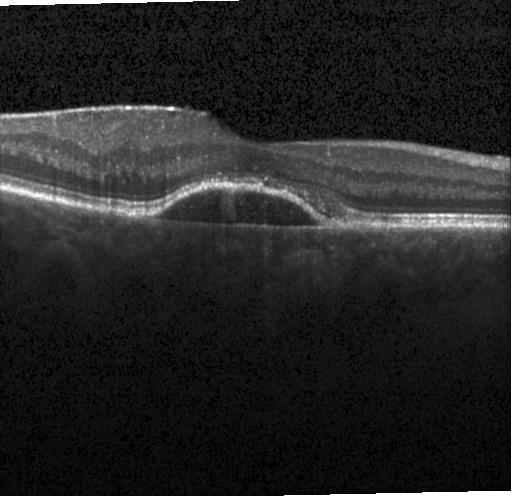

Retinal OCT B-scan, spectral-domain OCT, horizontal scan through the fovea, Heidelberg Spectralis OCT system. A choroidal neovascular membrane.